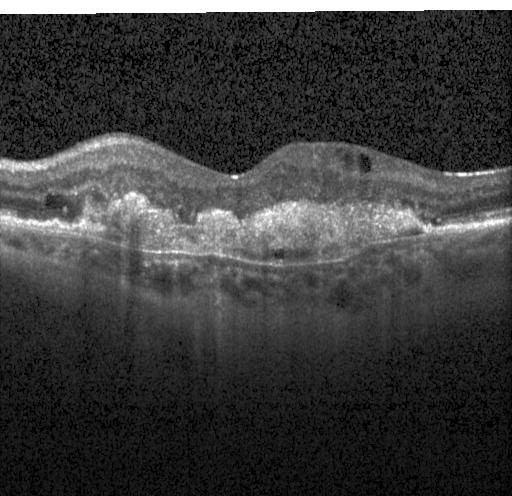 OCT line scan · Heidelberg Spectralis · centered on the fovea · SD-OCT
Macular OCT: a choroidal neovascular membrane.